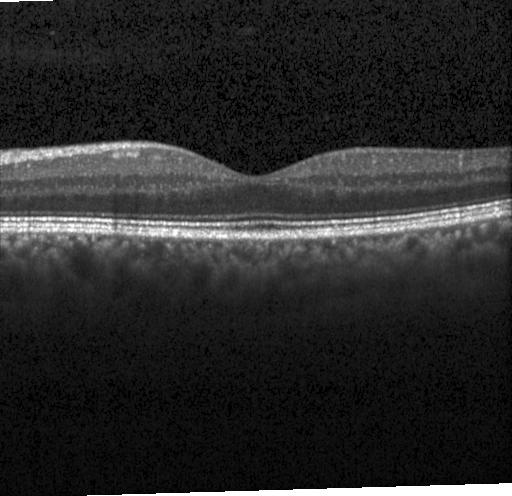 Instrument: Heidelberg Spectralis · optical coherence tomography scan · spectral-domain optical coherence tomography.
Assessment: no evidence of CNV, DME, or drusen.